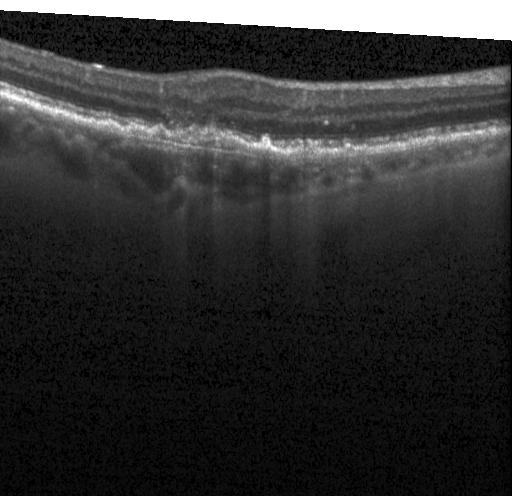 Optical coherence tomography B-scan. Diagnosis: a choroidal neovascular membrane.